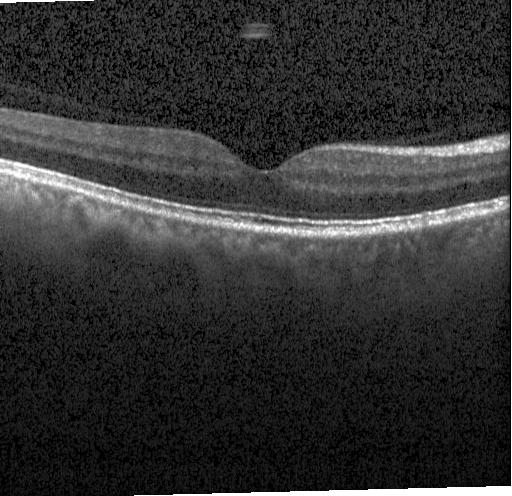

Spectral-domain OCT. OCT B-scan — Macular OCT: no choroidal neovascularization, diabetic macular edema, or drusen.